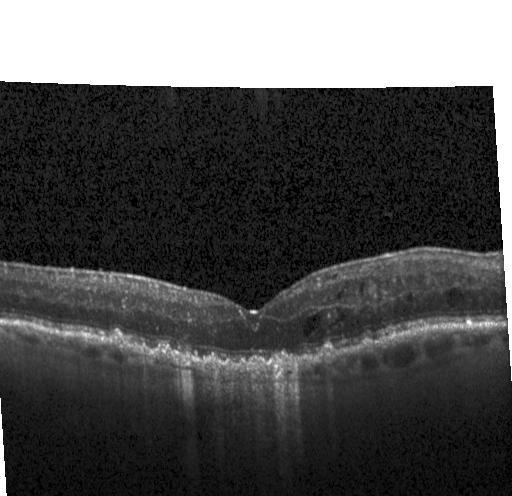 A choroidal neovascular membrane.